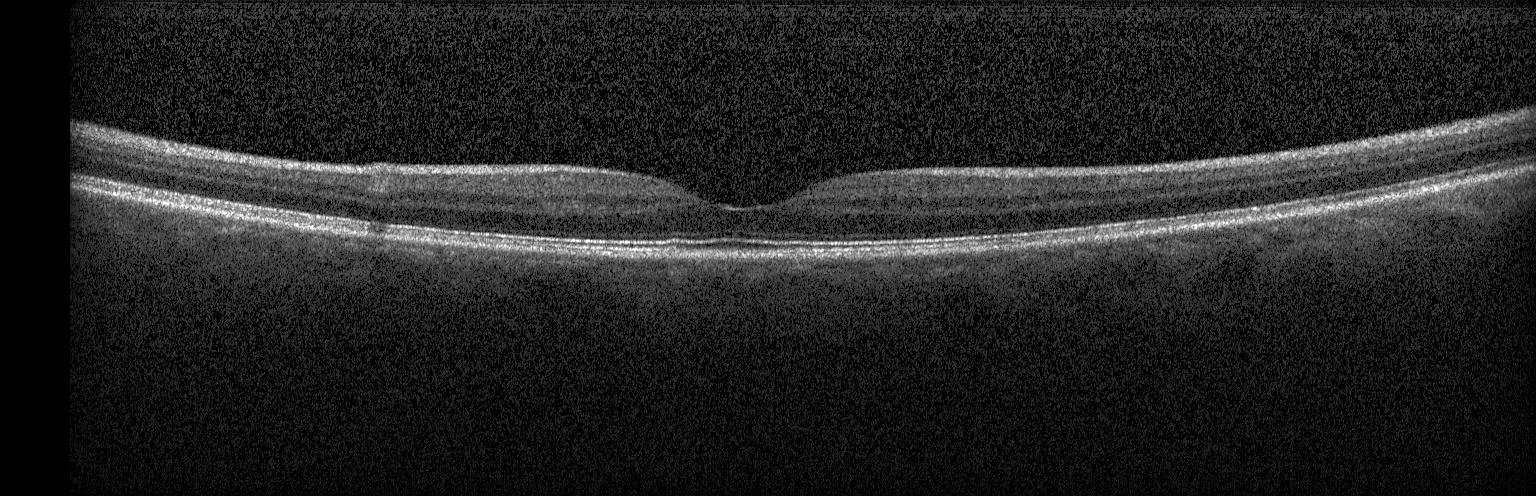

Spectral-domain OCT; OCT line scan — Assessment: no CNV, DME, or drusen.